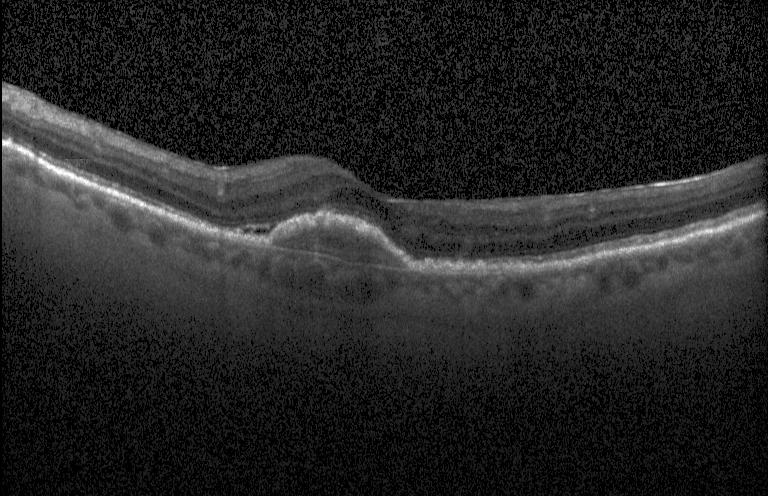
Through the macula. Optical coherence tomography B-scan. Instrument: Heidelberg Spectralis. Impression: a choroidal neovascular membrane.